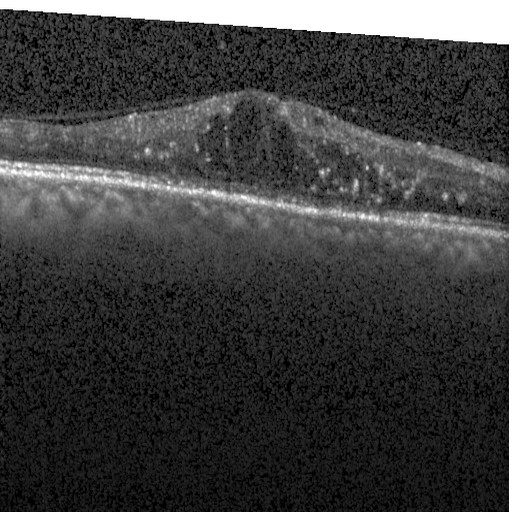

Optical coherence tomography B-scan, instrument: Heidelberg Spectralis
Diagnosis: diabetic macular edema (DME).